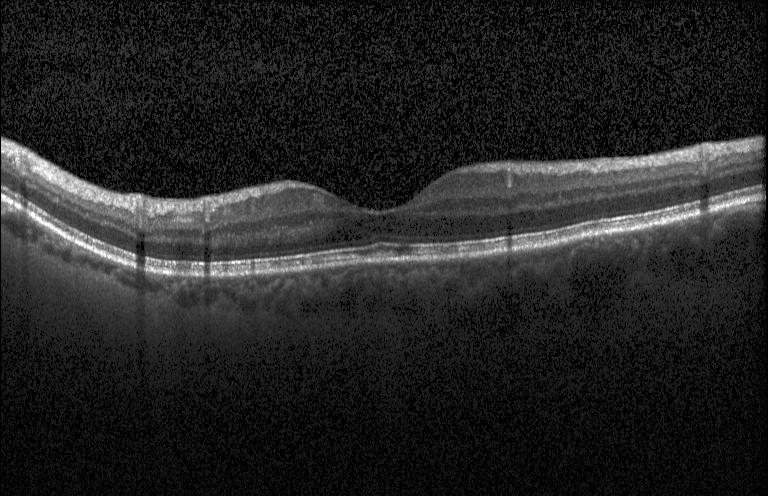
Optical coherence tomography B-scan, instrument: Heidelberg Spectralis. Diagnosis: no choroidal neovascularization, no diabetic macular edema, and no drusen.